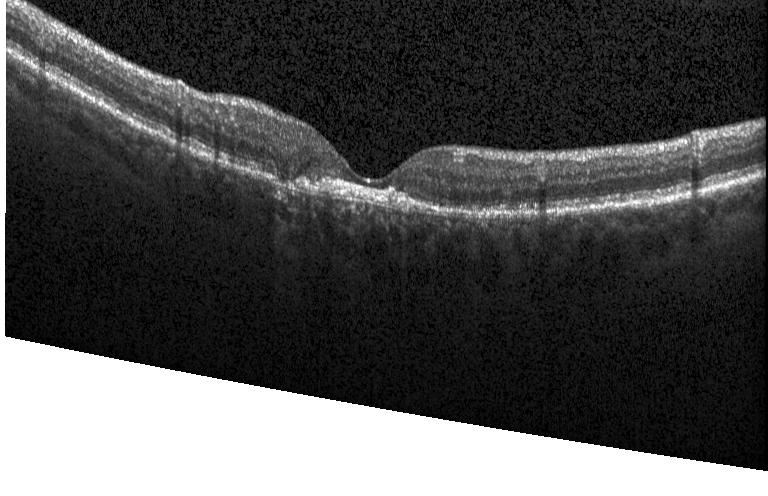
Spectral-domain optical coherence tomography. OCT B-scan.
Diagnosis: choroidal neovascularization.